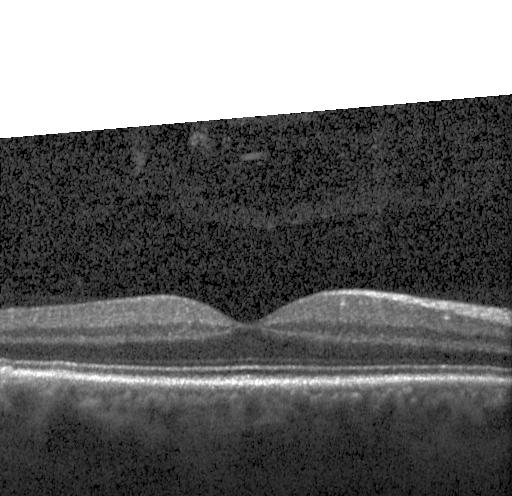
Macular OCT demonstrating neither choroidal neovascularization, diabetic macular edema, nor drusen.